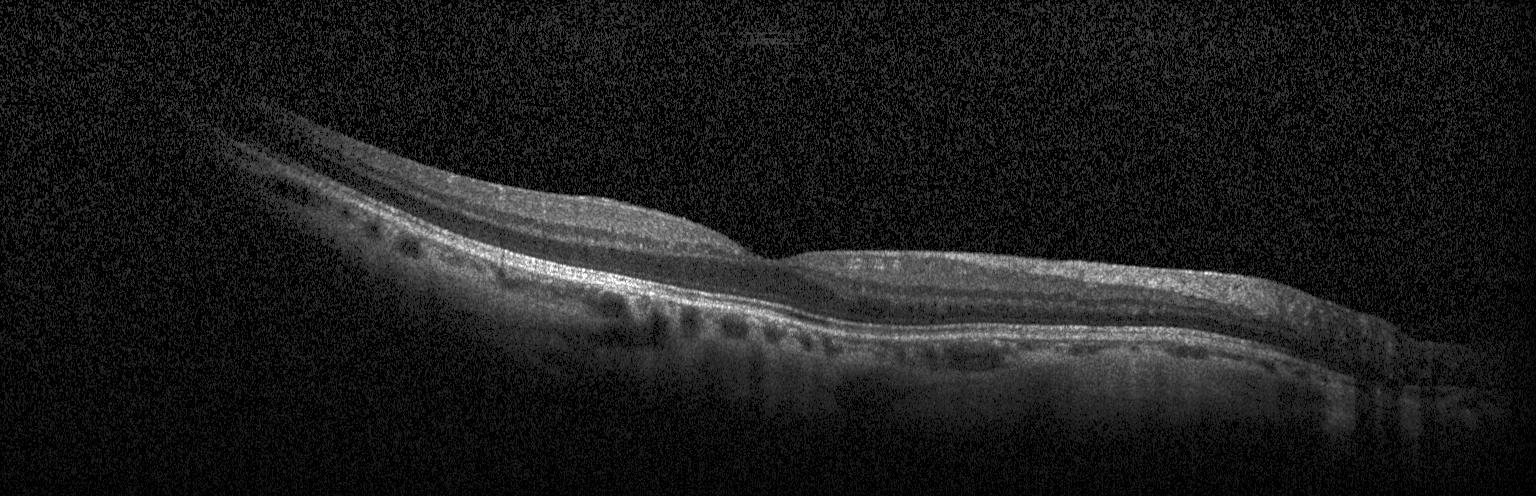
Macular scan · acquired on a Heidelberg Spectralis · retinal OCT B-scan
This B-scan demonstrates no CNV, no DME, and no drusen.